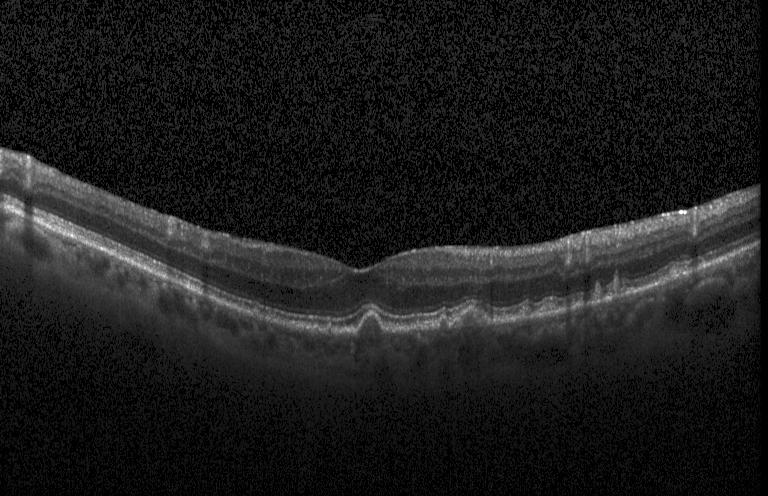

Optical coherence tomography scan — This B-scan demonstrates drusen.